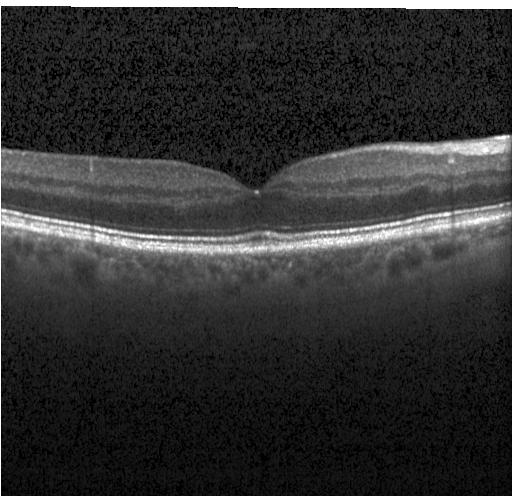
Spectral-domain OCT B-scan: neither CNV, DME, nor drusen.